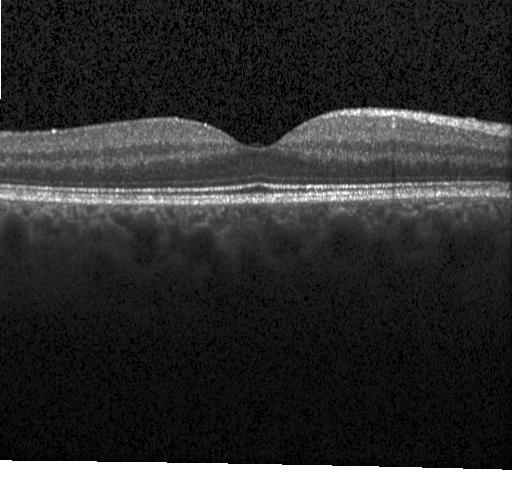 Finding: no choroidal neovascularization, diabetic macular edema, or drusen.